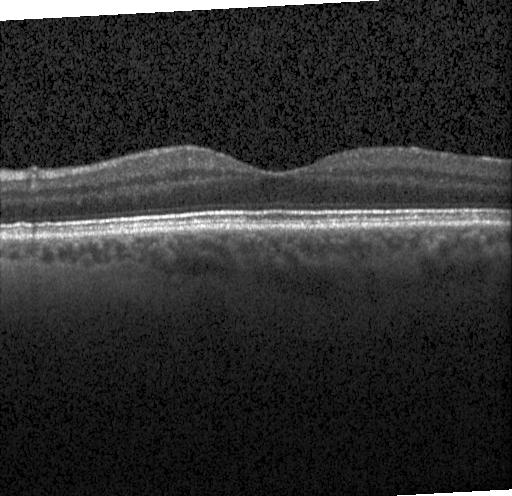 Retinal OCT cross-section · macular scan
Diagnosis: neither CNV, DME, nor drusen.